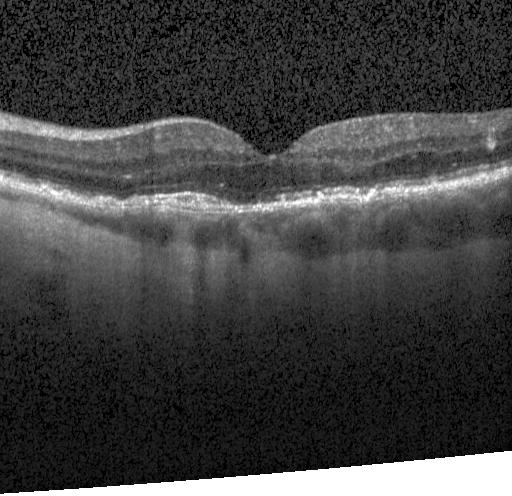

Retinal OCT B-scan.
Finding: a choroidal neovascular membrane.